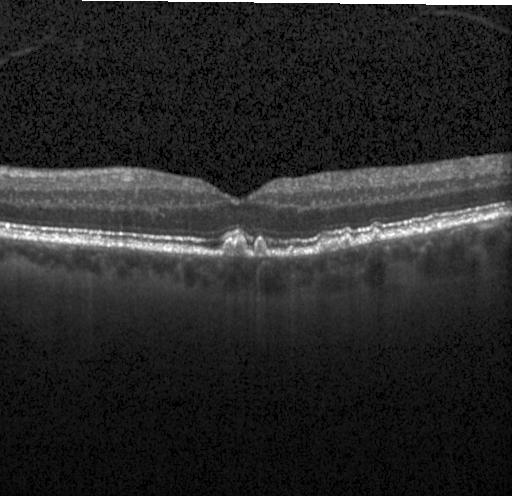 Impression: sub-RPE drusenoid deposits.